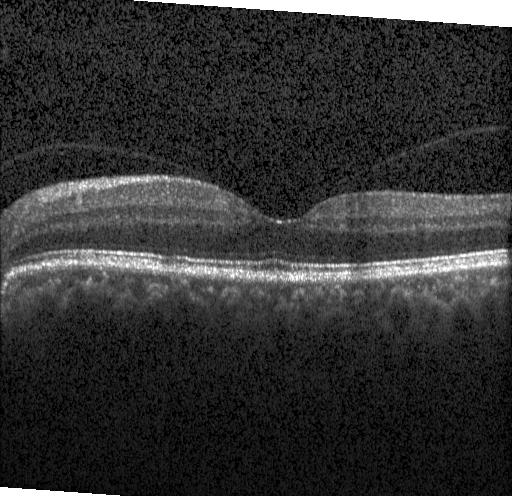

OCT B-scan. Finding: no CNV, no DME, and no drusen.